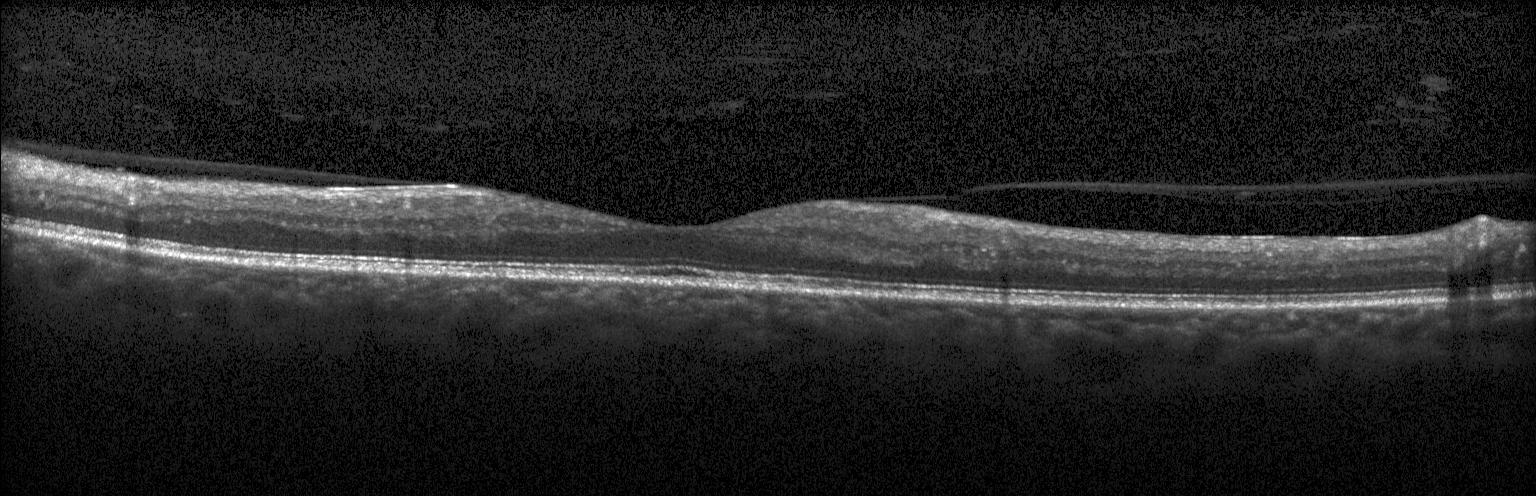

Assessment: no choroidal neovascularization, diabetic macular edema, or drusen.